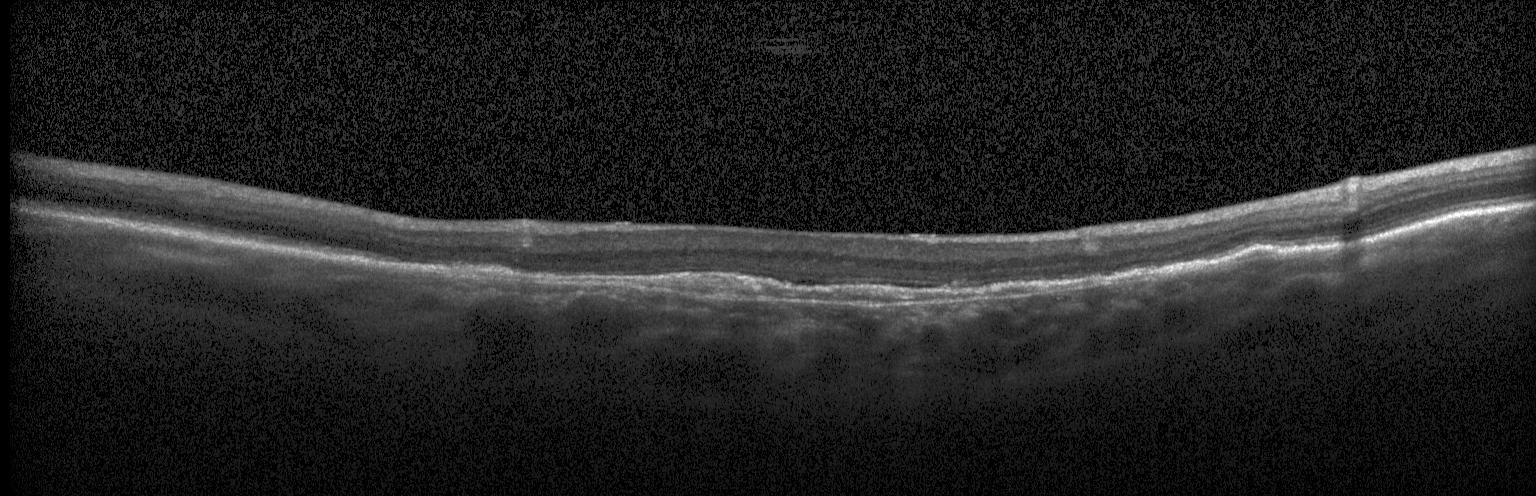

OCT B-scan showing a choroidal neovascular membrane.